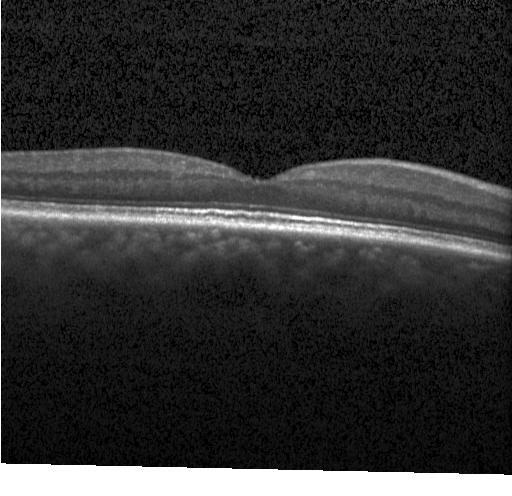

Retinal OCT cross-section.
OCT finding: neither choroidal neovascularization, diabetic macular edema, nor drusen.